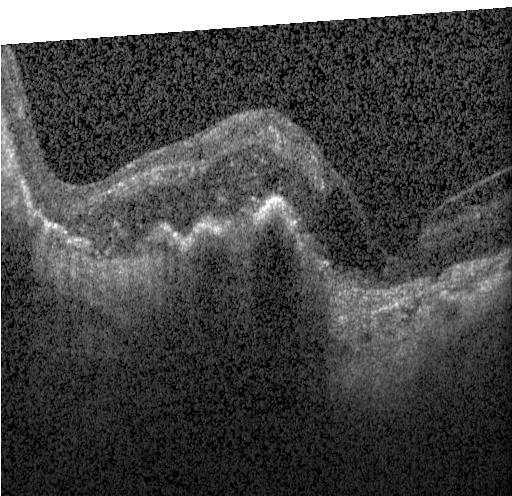 Choroidal neovascularization.